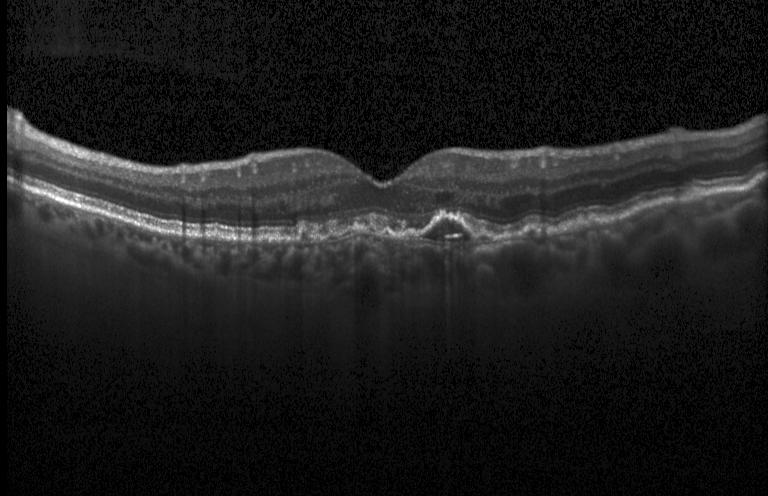 OCT line scan.
OCT finding: CNV.